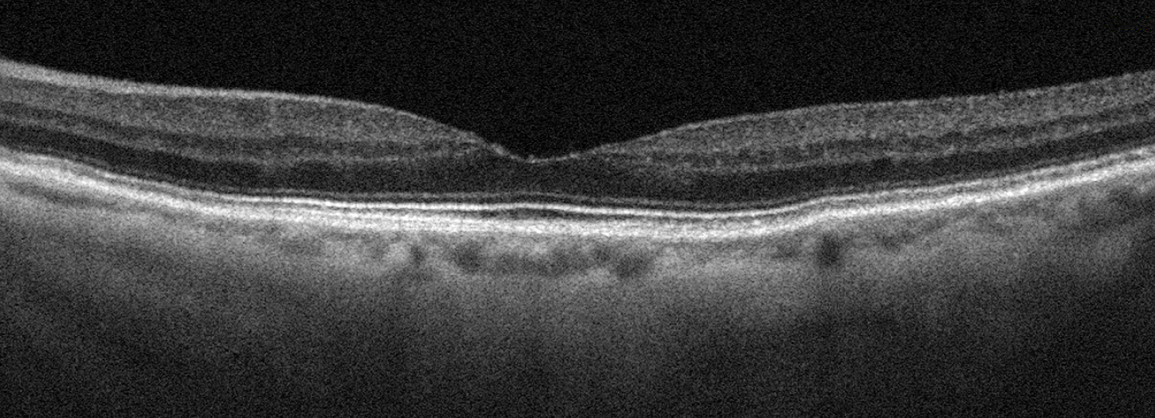

OCT B-scan · Optovue Avanti RTVue XR
Macular OCT: absence of AMD, DME, ERM, RAO, RVO, and vitreomacular interface disease.